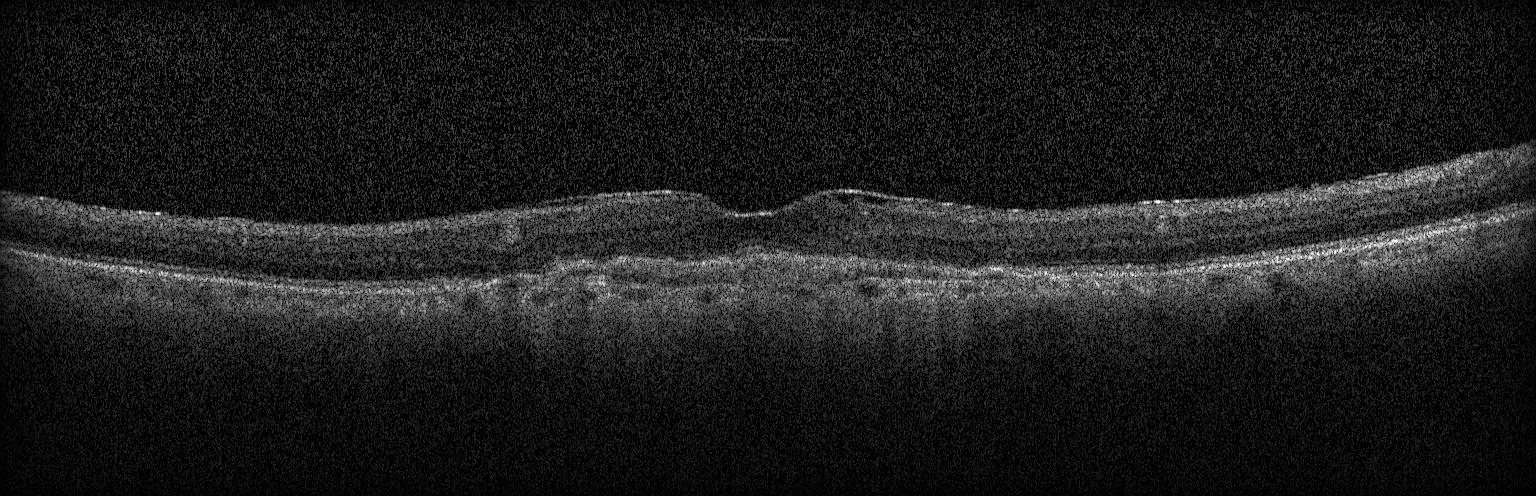

Retinal OCT cross-section
Choroidal neovascularization (CNV).